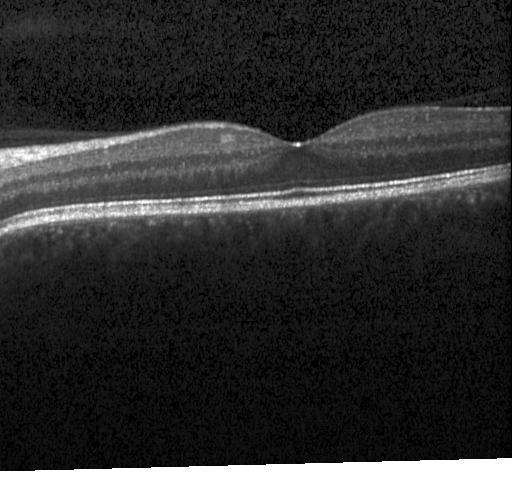 Optical coherence tomography scan
Impression: no choroidal neovascularization, diabetic macular edema, or drusen.